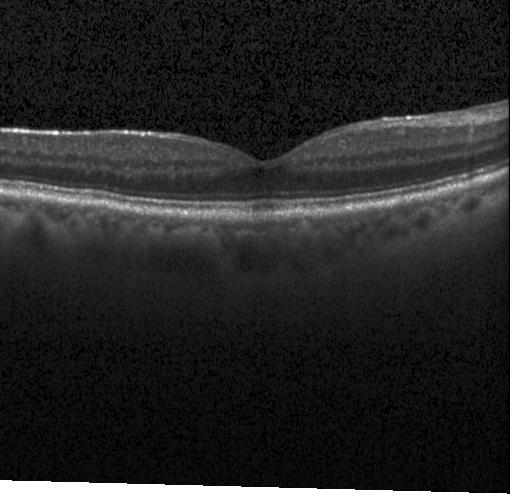 SD-OCT, OCT B-scan, centered on the fovea. Finding: neither CNV, DME, nor drusen.